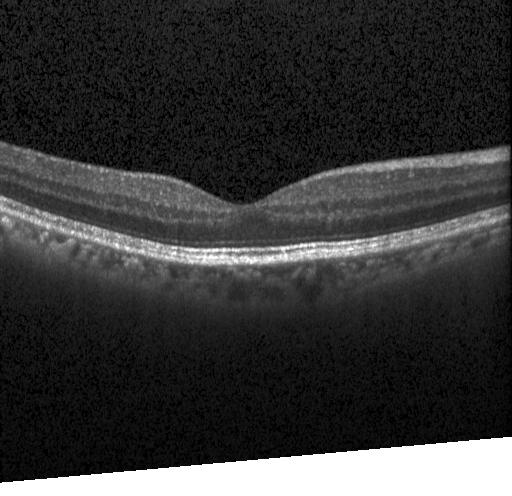

Optical coherence tomography B-scan — Diagnosis: no CNV, no DME, and no drusen.